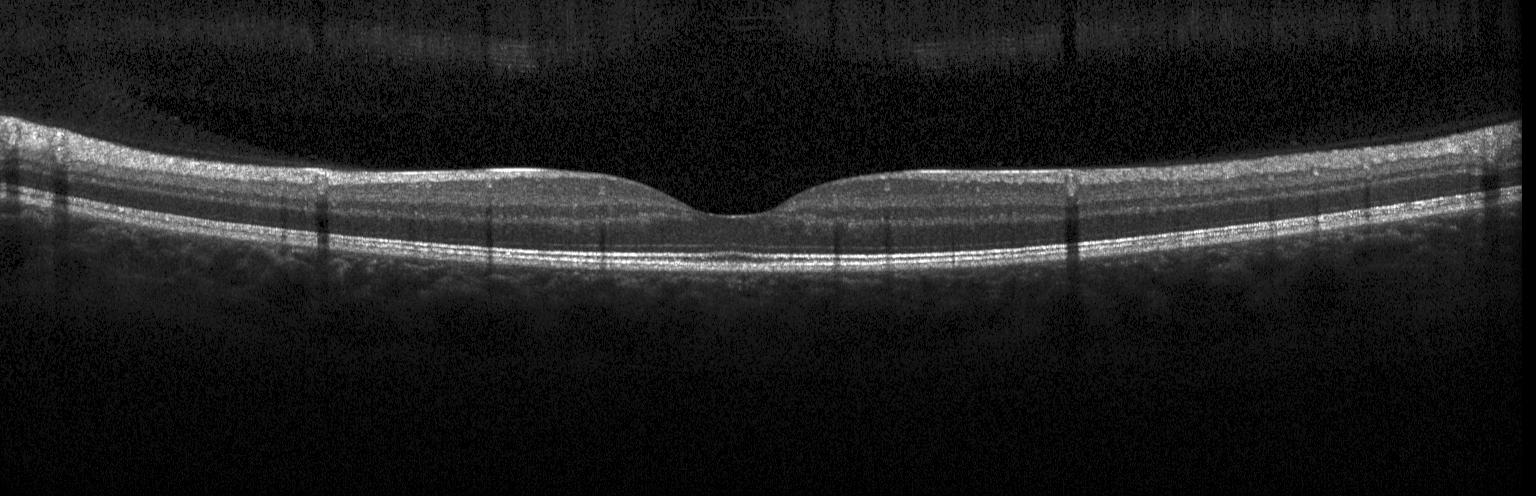
Retinal OCT B-scan
The scan shows neither choroidal neovascularization, diabetic macular edema, nor drusen.